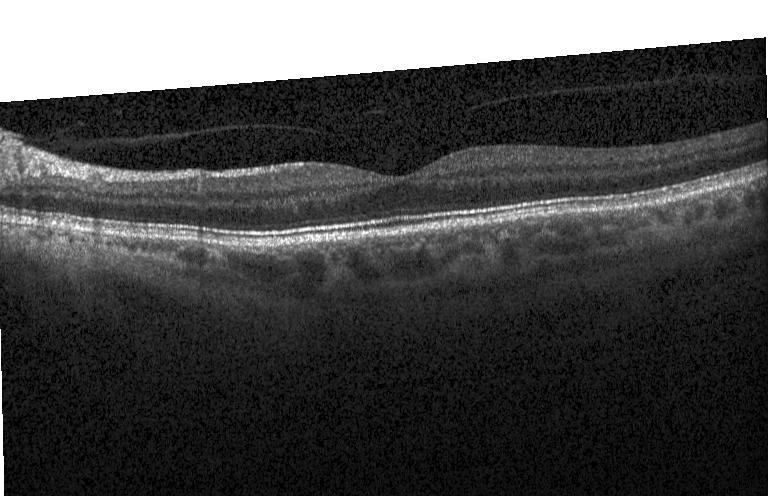

Heidelberg Spectralis · spectral-domain optical coherence tomography · retinal OCT B-scan · fovea-centered
Impression: neither choroidal neovascularization, diabetic macular edema, nor drusen.